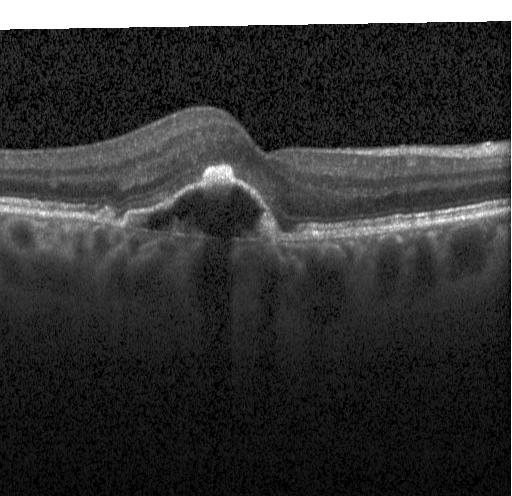

Horizontal scan through the fovea. OCT line scan
Diagnosis: choroidal neovascularization (CNV).